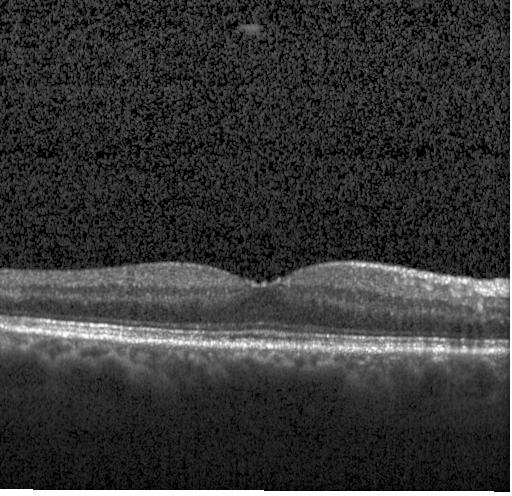 Spectral-domain OCT, acquired on a Heidelberg Spectralis, centered on the fovea, OCT line scan
The scan shows neither choroidal neovascularization, diabetic macular edema, nor drusen.